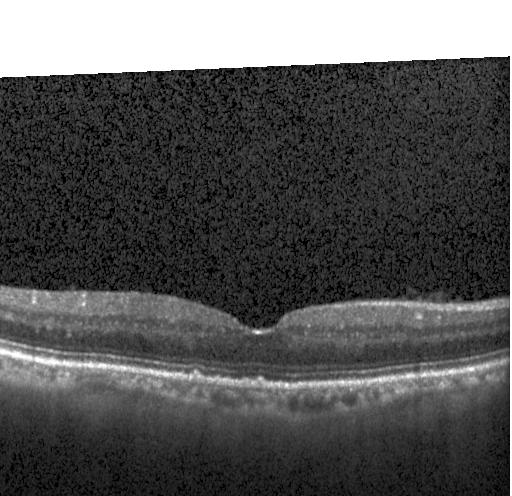 Retinal OCT cross-section, Heidelberg Spectralis, centered on the fovea, SD-OCT.
Sub-RPE drusenoid deposits.